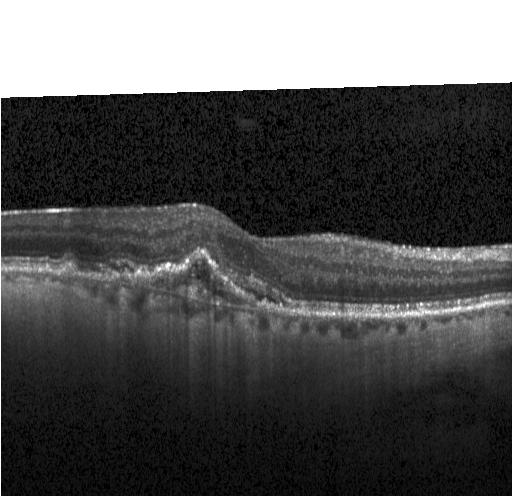

Retinal OCT B-scan.
A choroidal neovascular membrane.